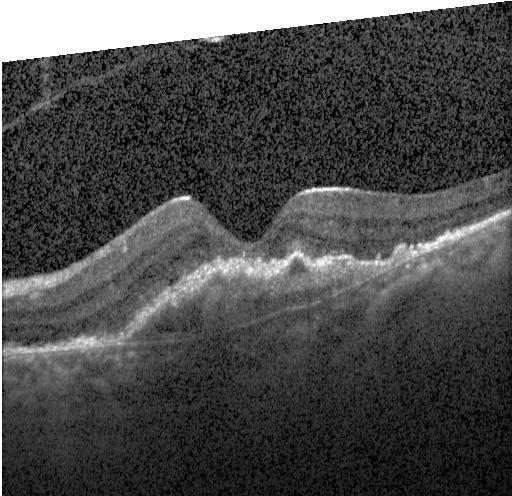
SD-OCT, fovea-centered, OCT line scan — Diagnosis: choroidal neovascularization (CNV).